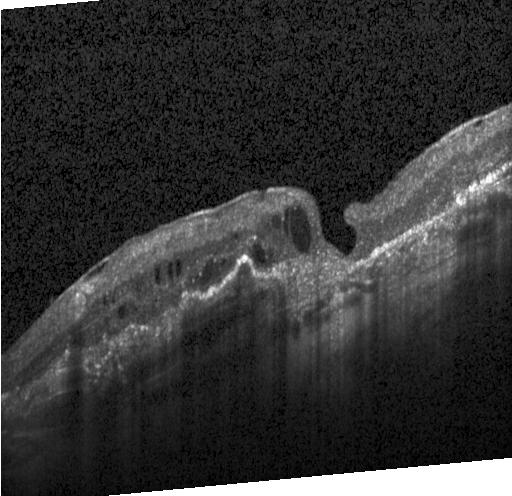

Horizontal scan through the fovea. OCT B-scan. Heidelberg Spectralis — Impression: choroidal neovascularization.